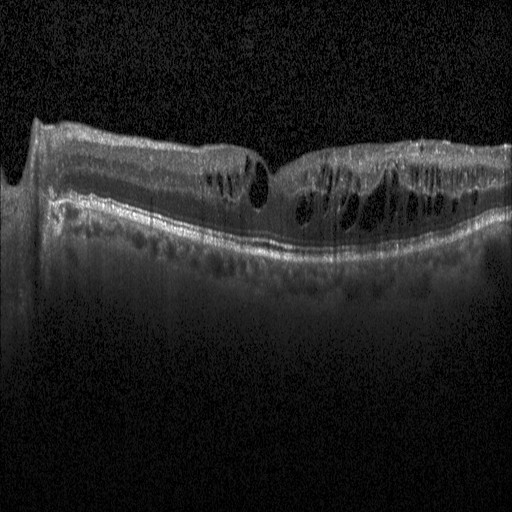

Optical coherence tomography B-scan. Spectral-domain OCT. Horizontal scan through the fovea. Heidelberg Spectralis.
Impression: diabetic macular edema (DME).